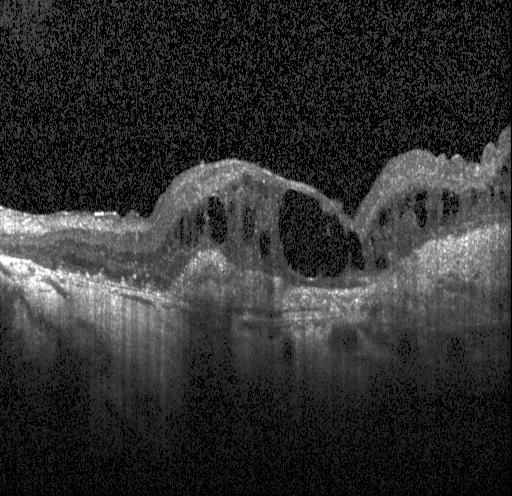
CNV.